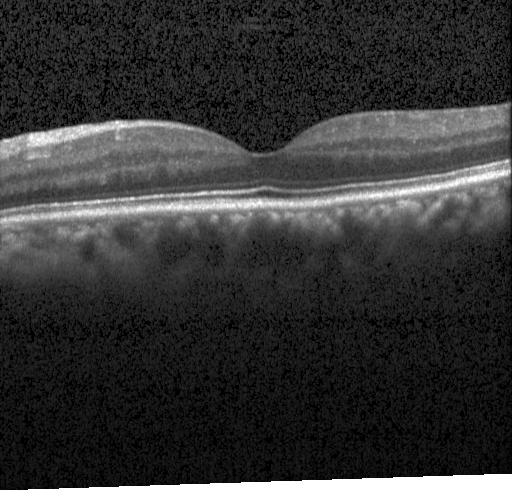 The scan shows no choroidal neovascularization, diabetic macular edema, or drusen.